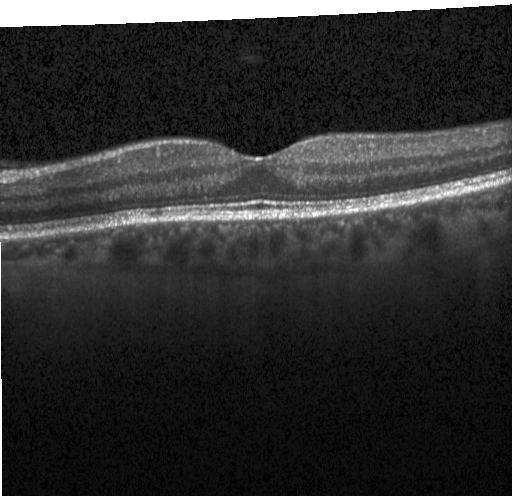

The scan shows no CNV, no DME, and no drusen.